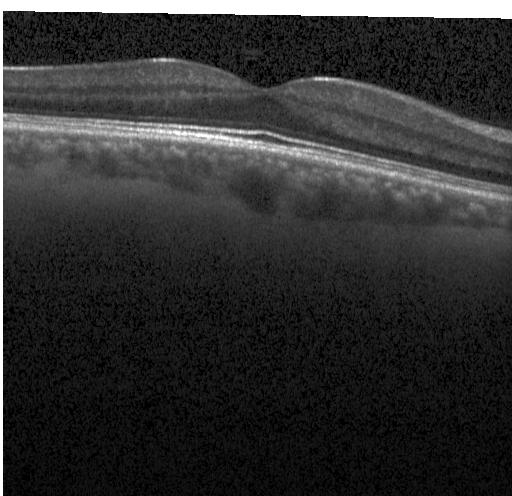 OCT line scan; through the macula
Assessment: neither choroidal neovascularization, diabetic macular edema, nor drusen.